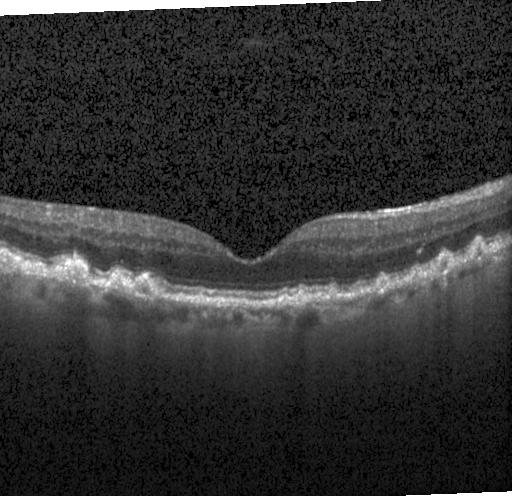

Spectral-domain optical coherence tomography, acquired on a Heidelberg Spectralis, retinal OCT cross-section, fovea-centered
Finding: multiple drusen.